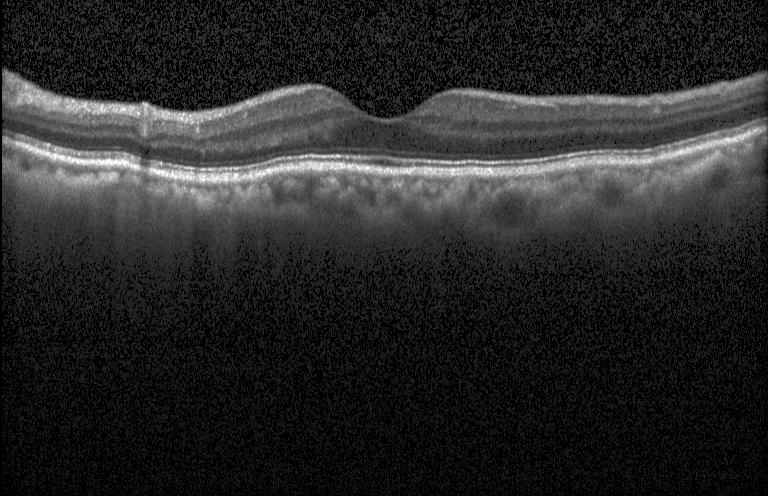
Assessment: no CNV, DME, or drusen.